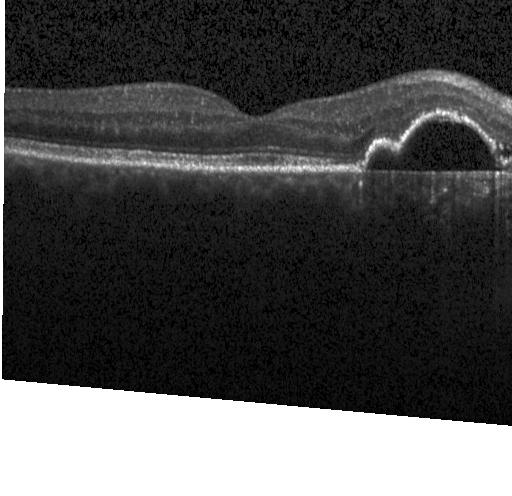
Finding: a choroidal neovascular membrane.